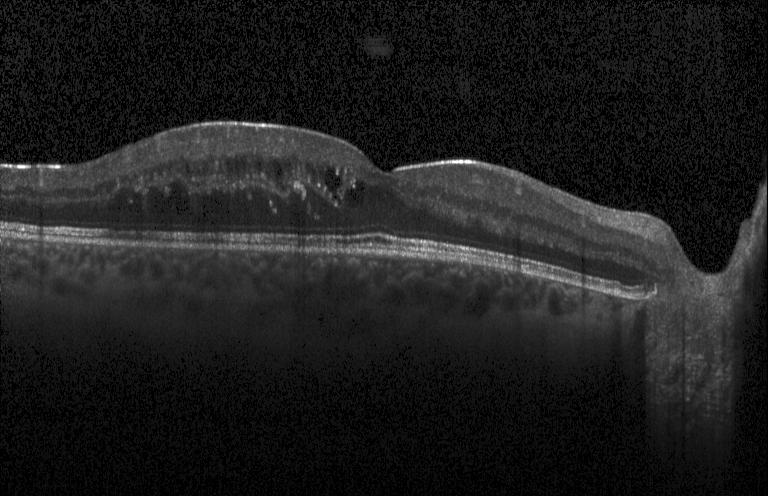
Spectral-domain optical coherence tomography, macular scan, OCT B-scan.
Impression: diabetic macular edema.